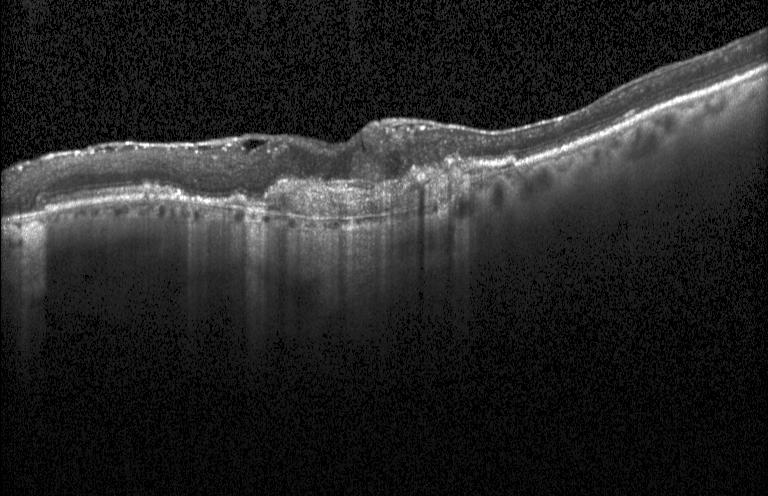 Retinal OCT B-scan · through the macula.
This B-scan demonstrates CNV.